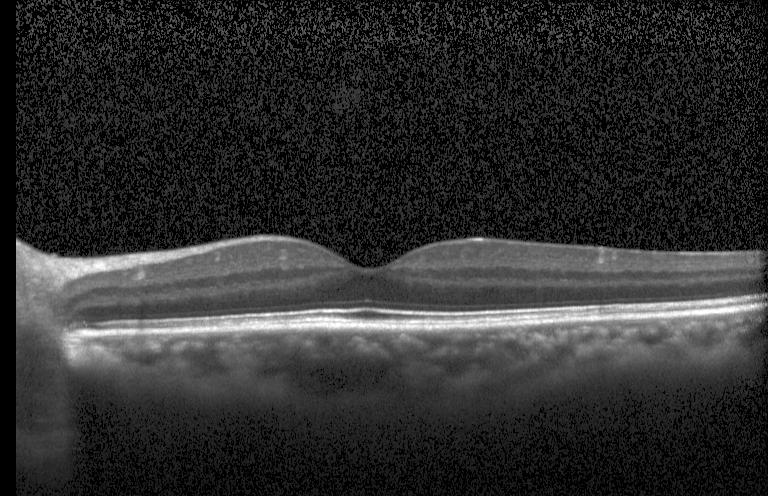

OCT scan showing neither CNV, DME, nor drusen.